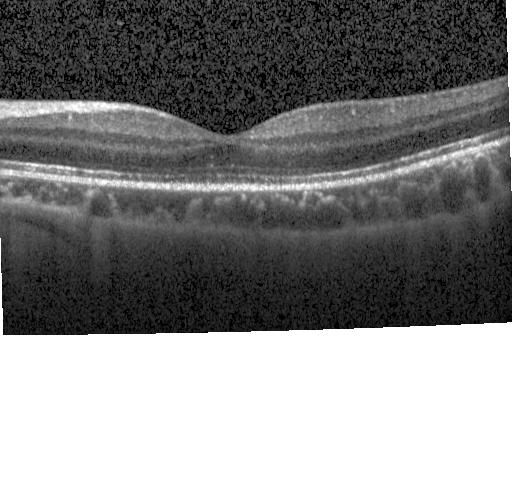

Retinal OCT cross-section showing no evidence of choroidal neovascularization, diabetic macular edema, or drusen.